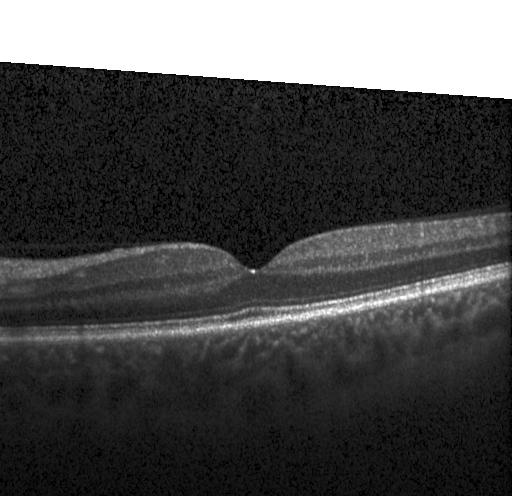

Centered on the fovea · spectral-domain optical coherence tomography · optical coherence tomography B-scan · instrument: Heidelberg Spectralis.
No choroidal neovascularization, diabetic macular edema, or drusen.